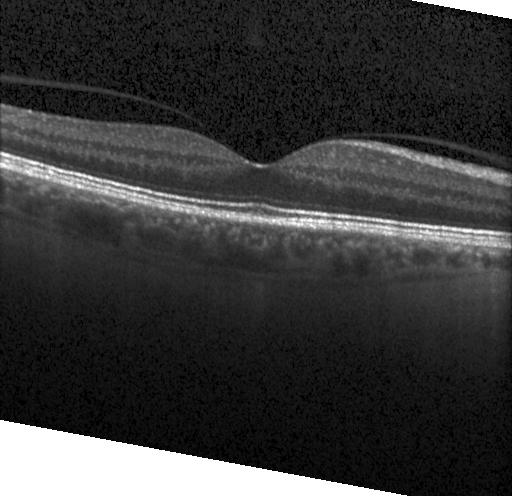
Assessment: neither CNV, DME, nor drusen.